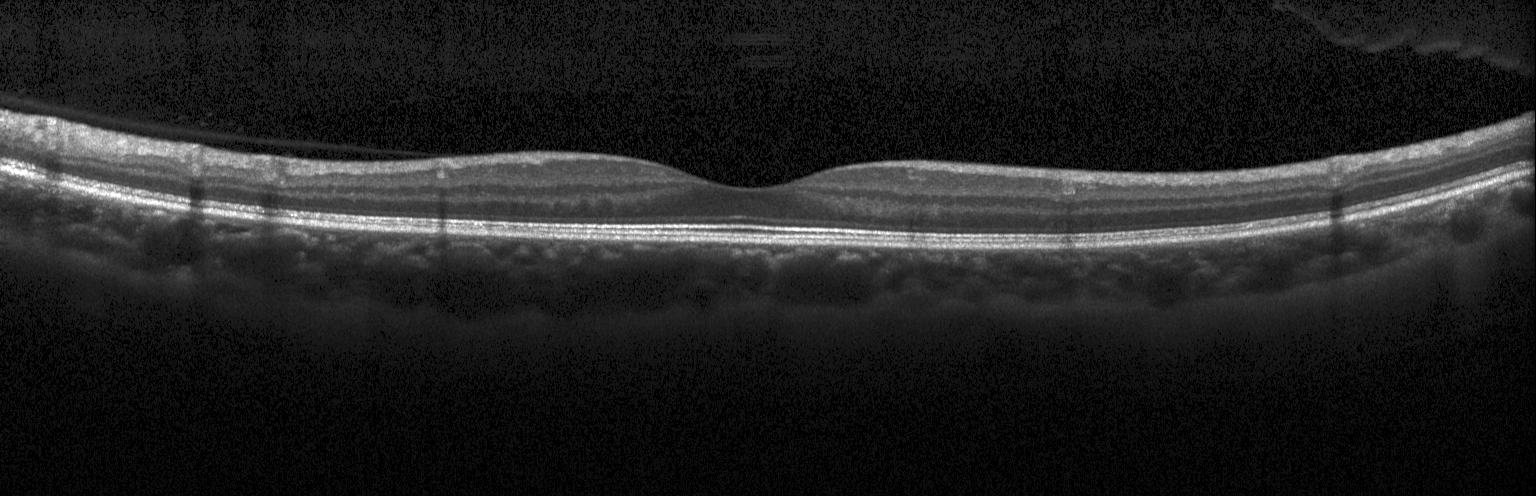 Centered on the fovea · spectral-domain optical coherence tomography · retinal OCT B-scan · Heidelberg Spectralis.
Assessment: no choroidal neovascularization, no diabetic macular edema, and no drusen.